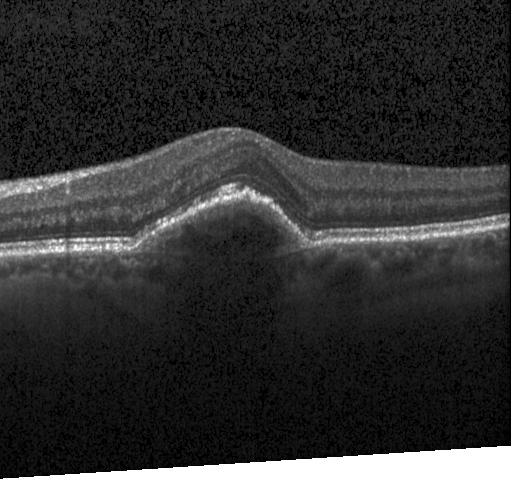
OCT line scan; spectral-domain OCT; fovea-centered. Choroidal neovascularization (CNV).